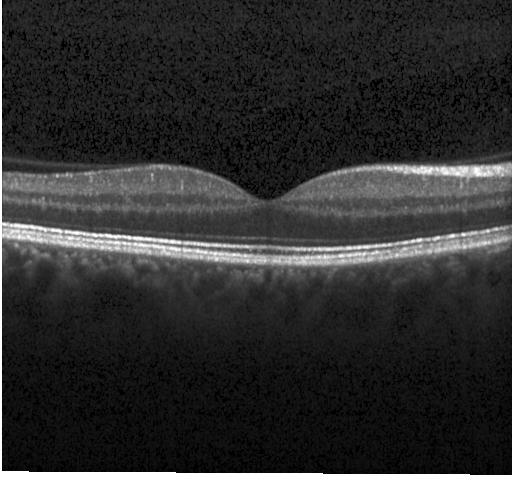
Heidelberg Spectralis · spectral-domain OCT · OCT B-scan · through the macula
Finding: no evidence of choroidal neovascularization, diabetic macular edema, or drusen.